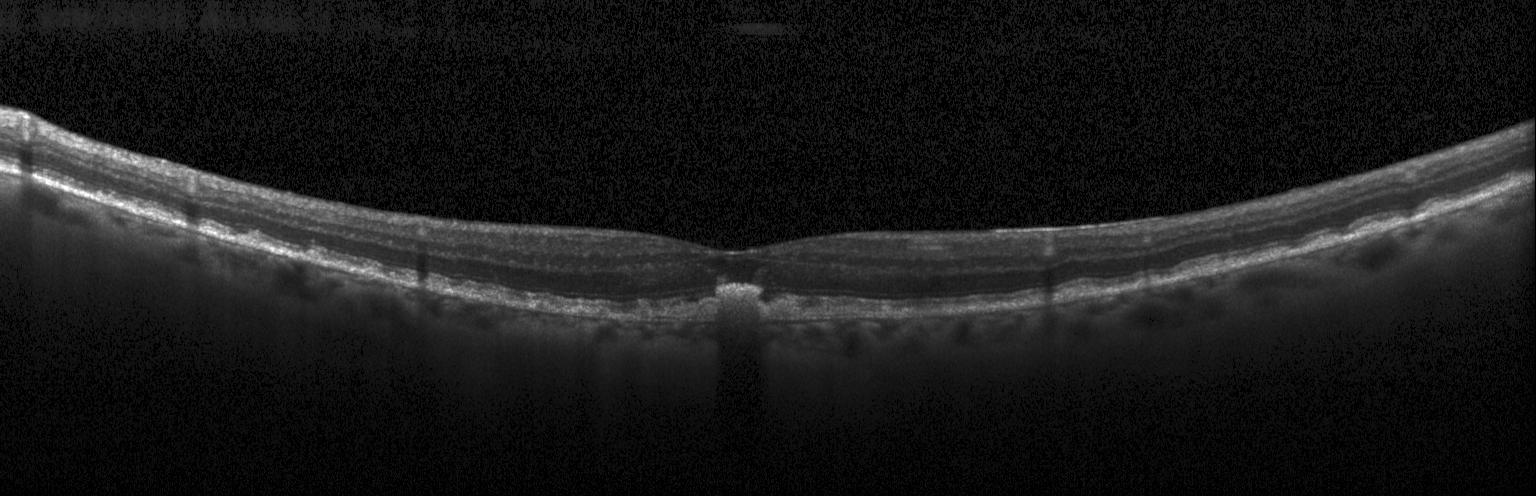

Optical coherence tomography scan. Drusen.